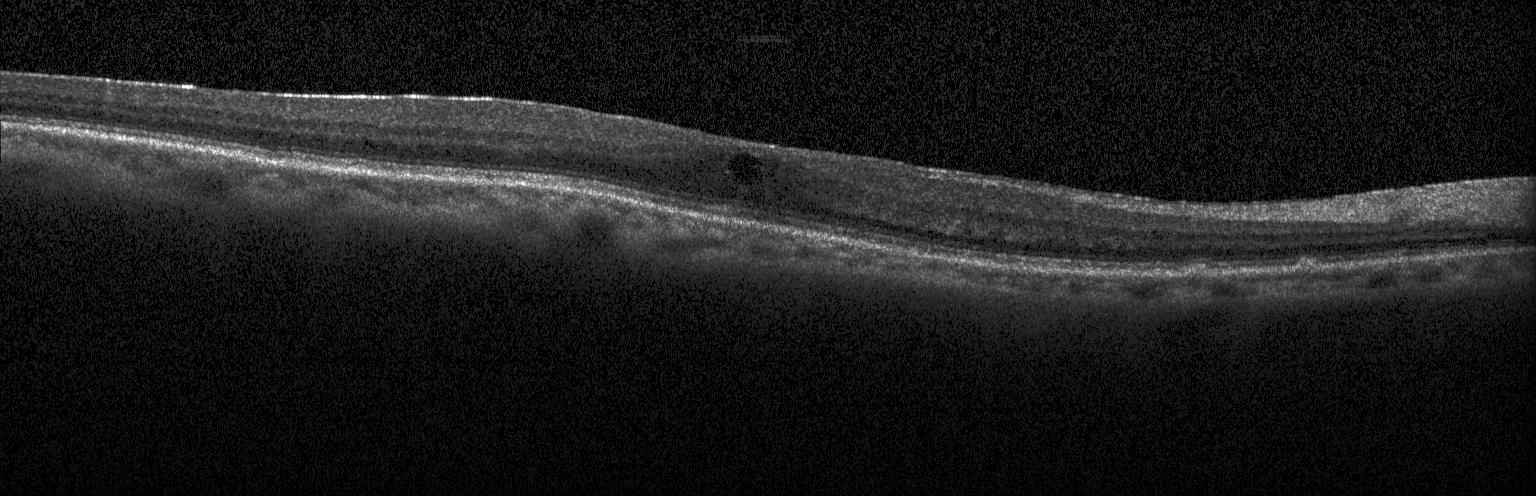 Finding: diabetic macular edema (DME).